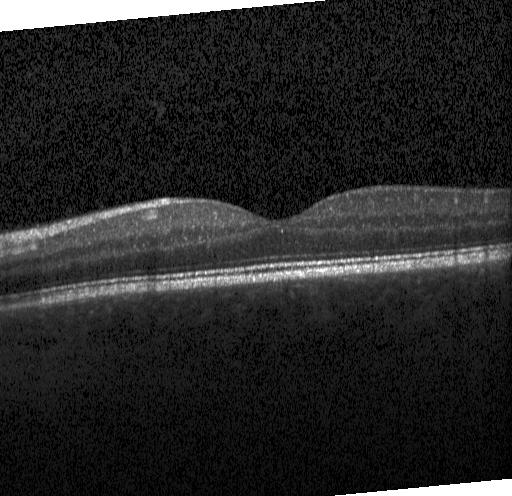

Through the macula · acquired on a Heidelberg Spectralis · SD-OCT · OCT B-scan. OCT finding: no evidence of choroidal neovascularization, diabetic macular edema, or drusen.